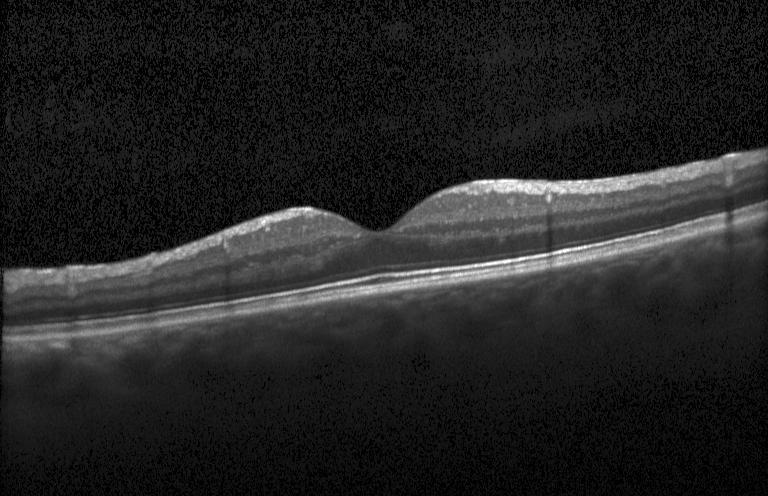 Optical coherence tomography B-scan. Centered on the fovea. Acquired on a Heidelberg Spectralis.
Finding: no choroidal neovascularization, diabetic macular edema, or drusen.